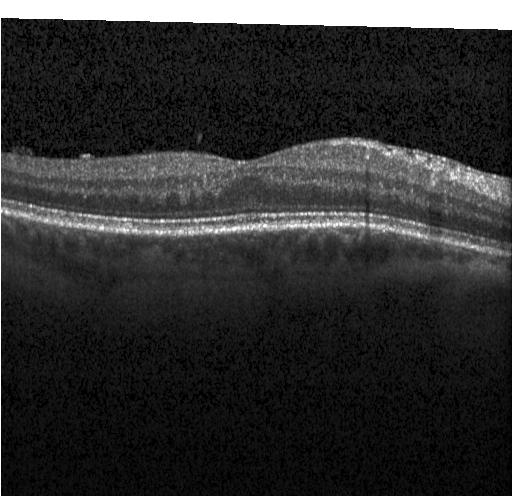 Retinal OCT cross-section · acquired on a Heidelberg Spectralis.
Impression: neither choroidal neovascularization, diabetic macular edema, nor drusen.